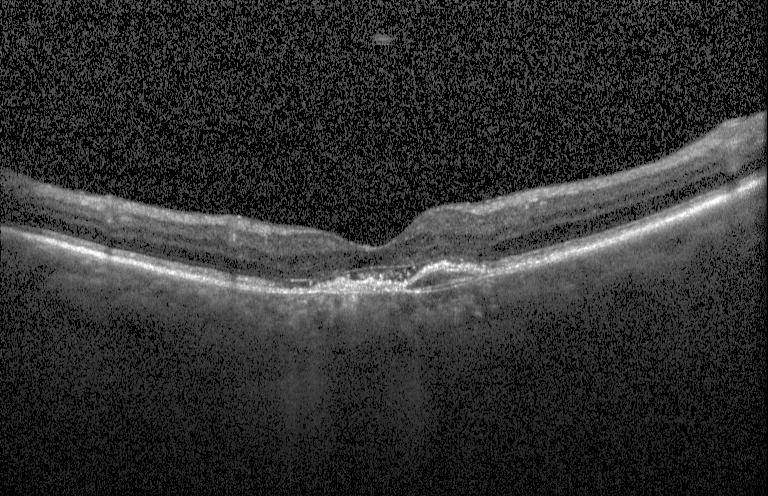 OCT B-scan.
Impression: choroidal neovascularization (CNV).